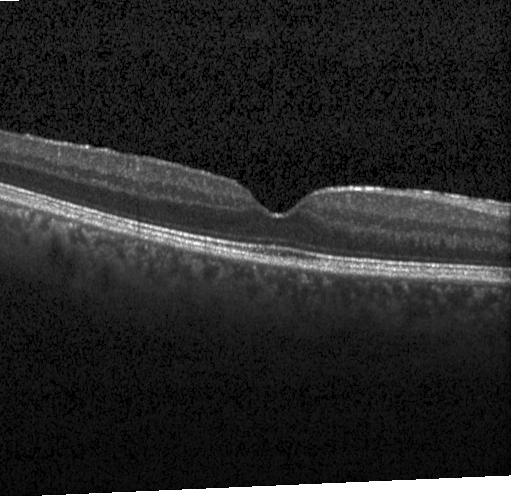

Retinal OCT B-scan. Spectral-domain OCT. Finding: neither choroidal neovascularization, diabetic macular edema, nor drusen.